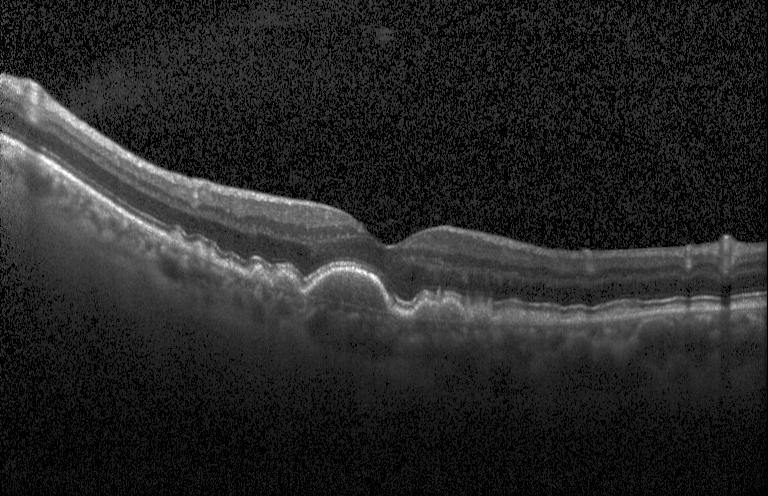
OCT line scan, through the macula.
Impression: multiple drusen.